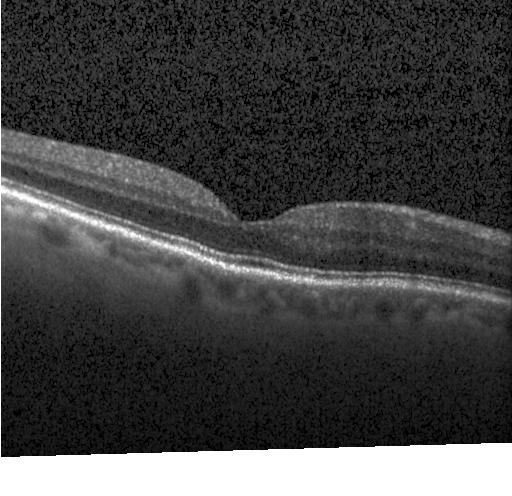

No choroidal neovascularization, no diabetic macular edema, and no drusen.